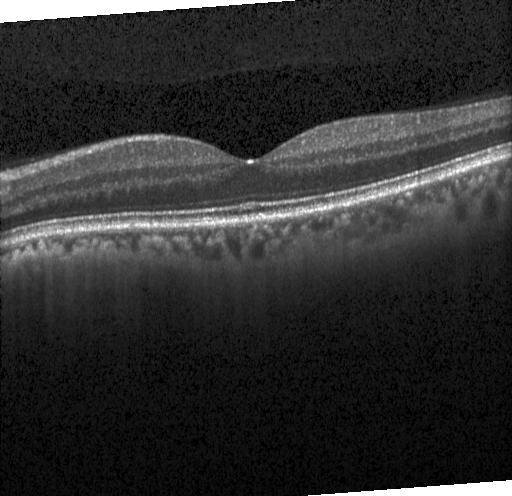
Impression: no choroidal neovascularization, no diabetic macular edema, and no drusen.